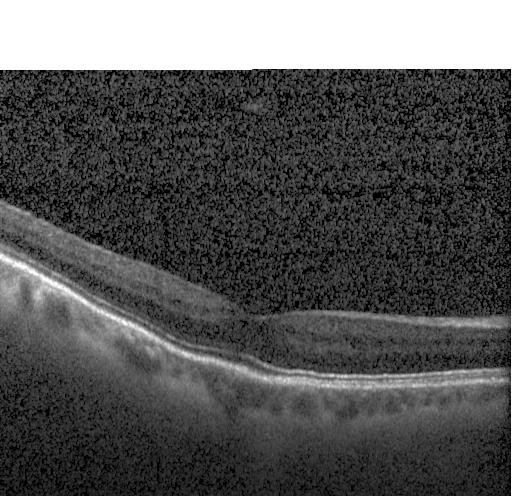 Neither choroidal neovascularization, diabetic macular edema, nor drusen.